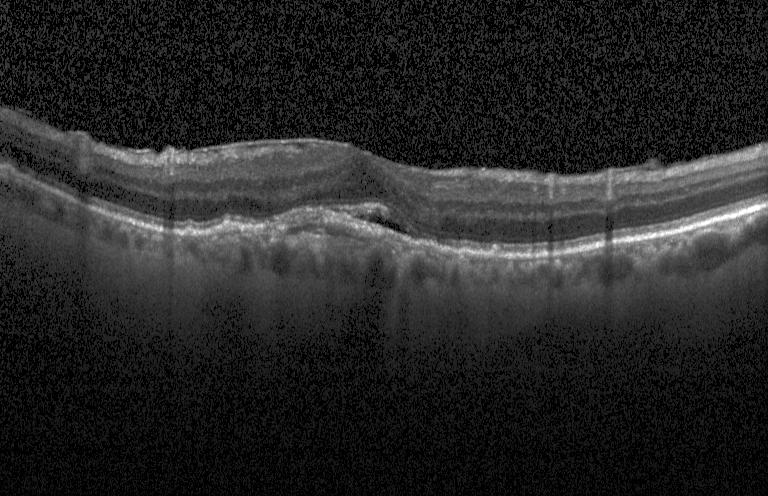 Heidelberg Spectralis OCT system · retinal OCT B-scan · fovea-centered
Diagnosis: a choroidal neovascular membrane.